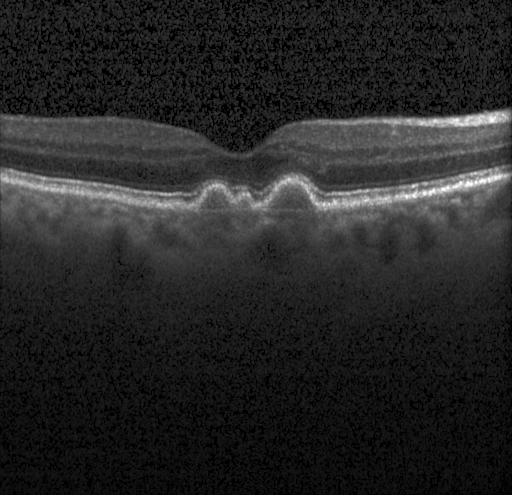

SD-OCT, retinal OCT cross-section — This B-scan demonstrates drusen.